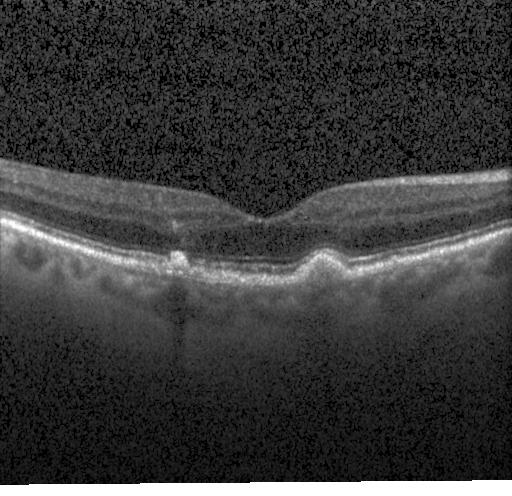 Spectral-domain OCT B-scan: multiple drusen.